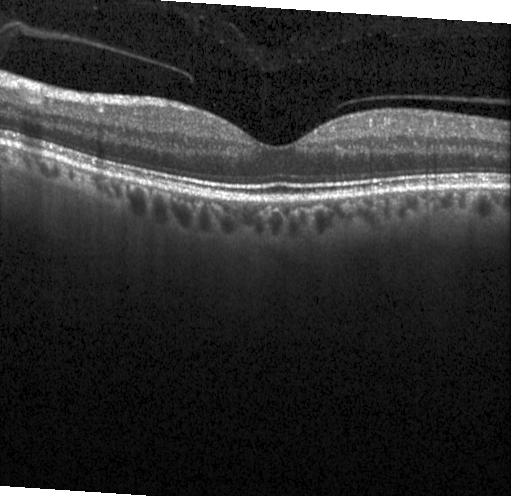

Spectral-domain OCT. Optical coherence tomography B-scan.
Macular OCT: no CNV, no DME, and no drusen.